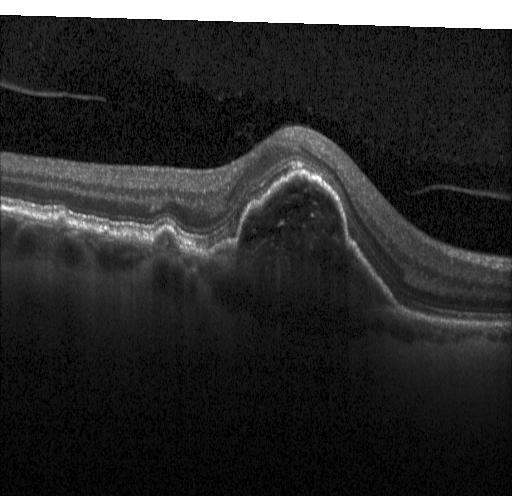

Optical coherence tomography scan
Impression: choroidal neovascularization (CNV).